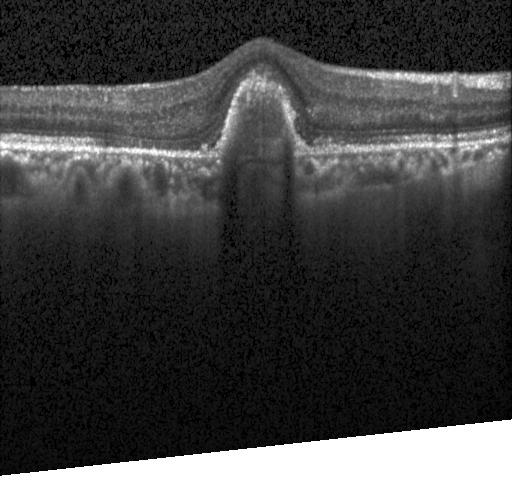 Heidelberg Spectralis · SD-OCT · optical coherence tomography scan
Diagnosis: choroidal neovascularization.